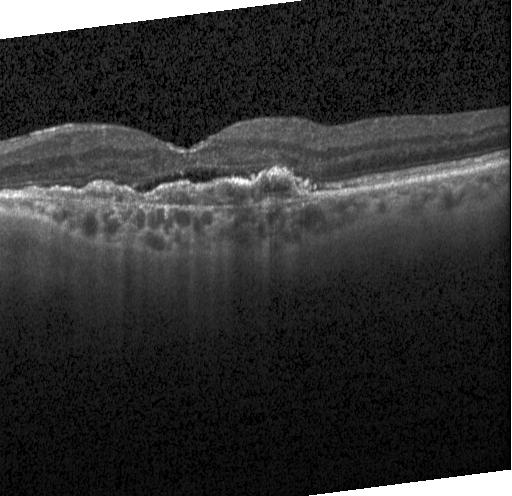 Spectral-domain optical coherence tomography, instrument: Heidelberg Spectralis, optical coherence tomography scan — Finding: a choroidal neovascular membrane.